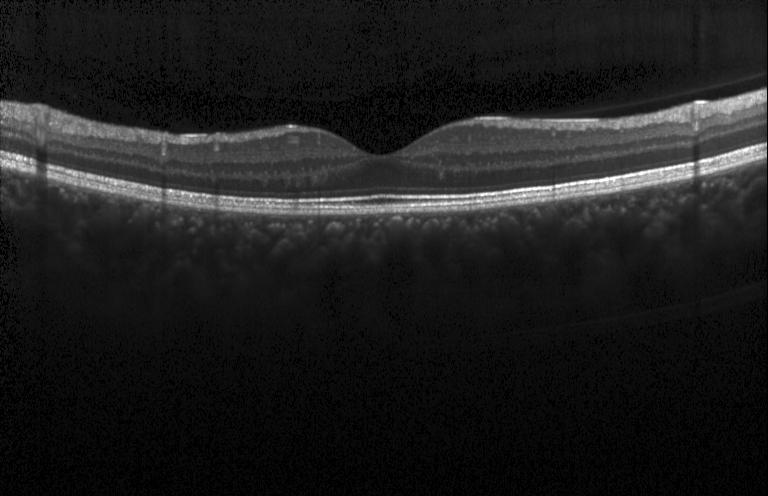

Acquired on a Heidelberg Spectralis, spectral-domain OCT, optical coherence tomography B-scan, centered on the fovea
Diagnosis: no evidence of choroidal neovascularization, diabetic macular edema, or drusen.